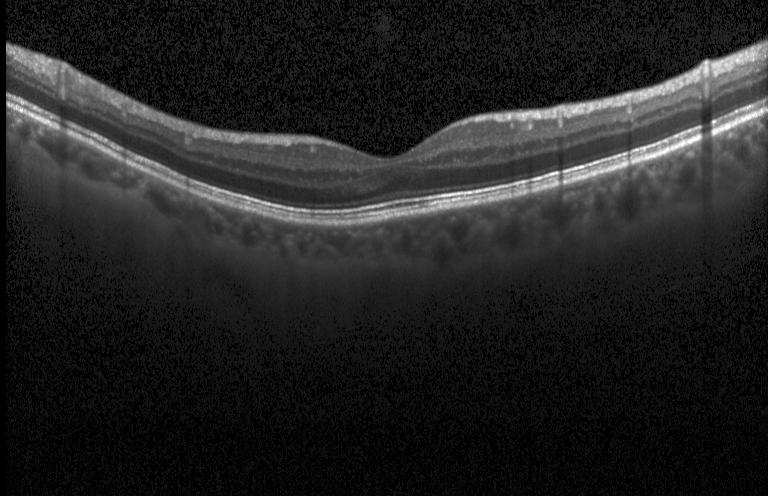
Retinal OCT B-scan.
Impression: neither CNV, DME, nor drusen.